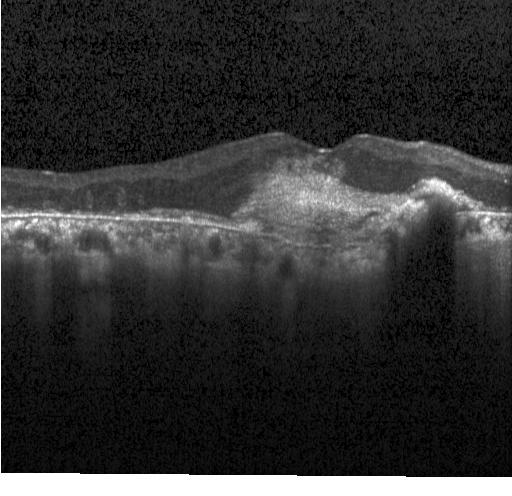
Spectral-domain OCT; centered on the fovea; OCT line scan; acquired on a Heidelberg Spectralis. Diagnosis: a choroidal neovascular membrane.